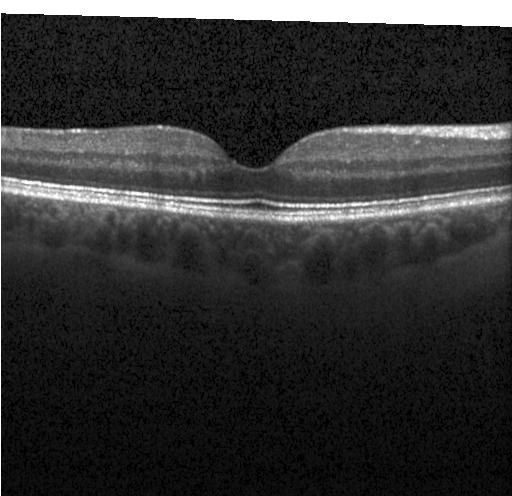

Finding: no evidence of choroidal neovascularization, diabetic macular edema, or drusen.